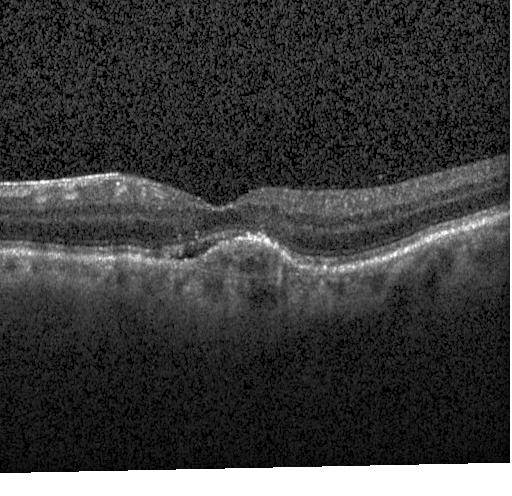
The scan shows a choroidal neovascular membrane.